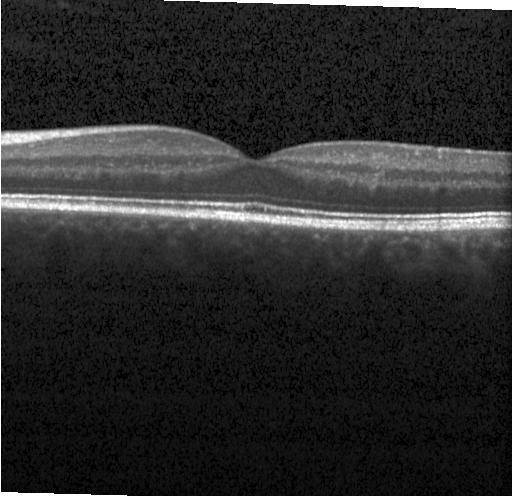 Retinal OCT cross-section, horizontal scan through the fovea — Dx: no CNV, no DME, and no drusen.